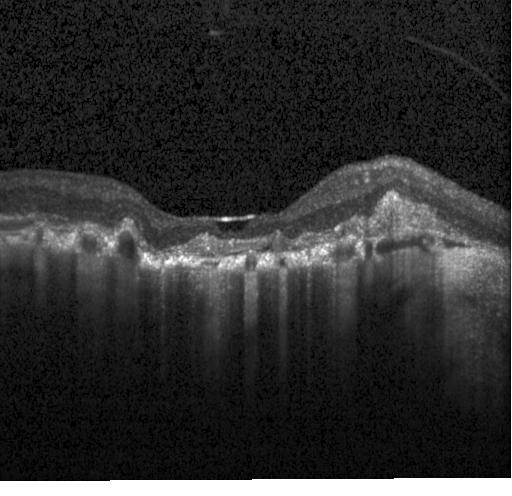

SD-OCT · retinal OCT B-scan
This B-scan demonstrates a choroidal neovascular membrane.